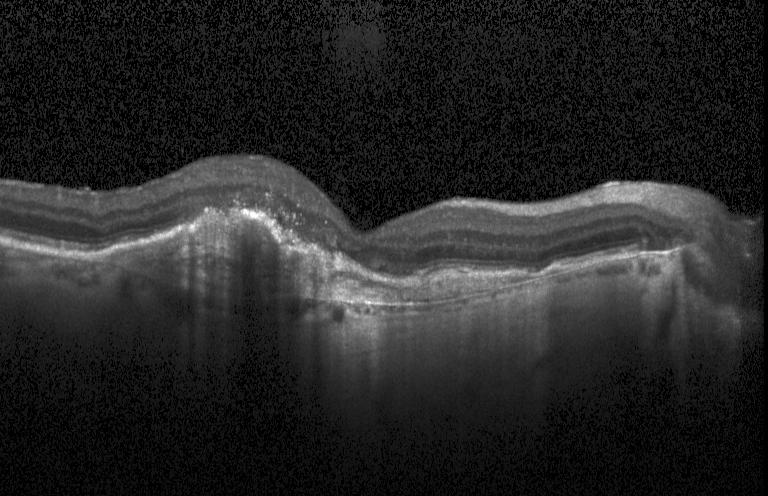
Diagnosis: a choroidal neovascular membrane.